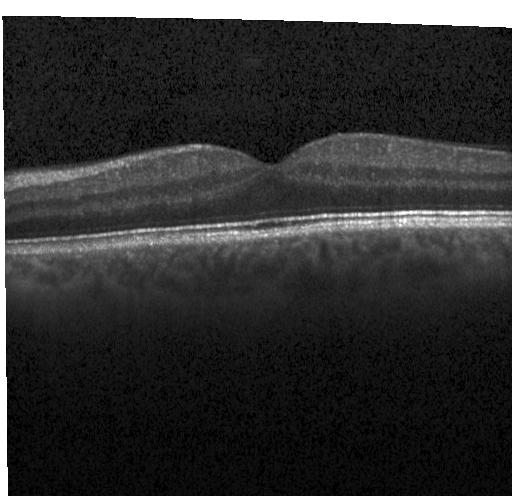
OCT finding: no choroidal neovascularization, no diabetic macular edema, and no drusen.